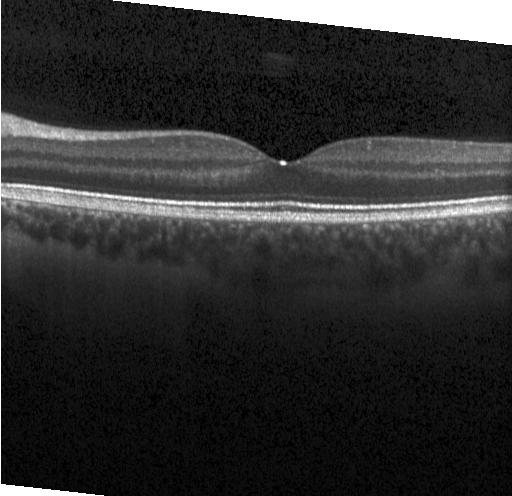

Impression: no choroidal neovascularization, diabetic macular edema, or drusen.